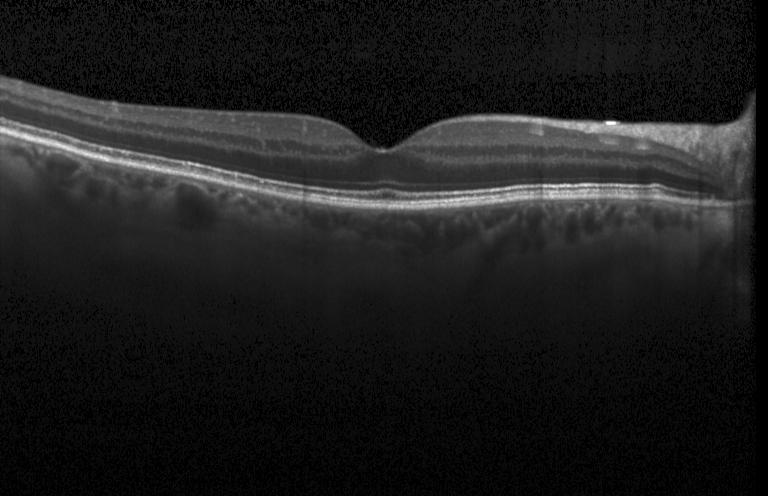 The scan shows no evidence of choroidal neovascularization, diabetic macular edema, or drusen.